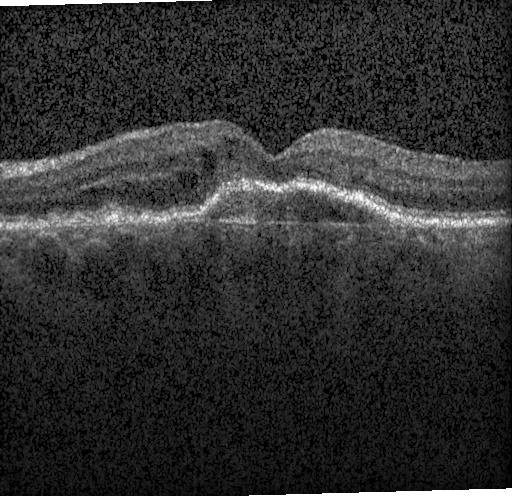 Optical coherence tomography scan, spectral-domain optical coherence tomography, Heidelberg Spectralis
Assessment: CNV.